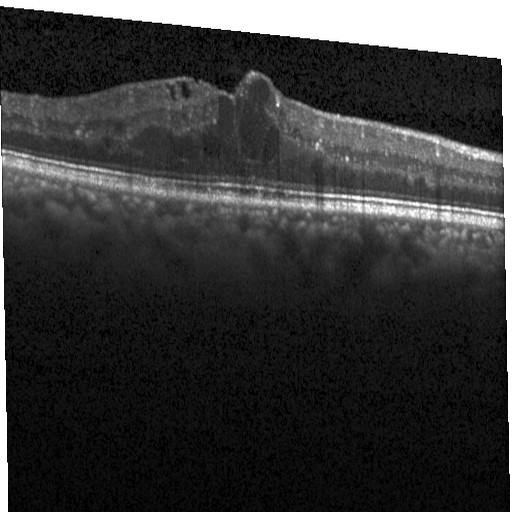

Heidelberg Spectralis OCT system · spectral-domain OCT · optical coherence tomography B-scan. The scan shows diabetic macular edema.